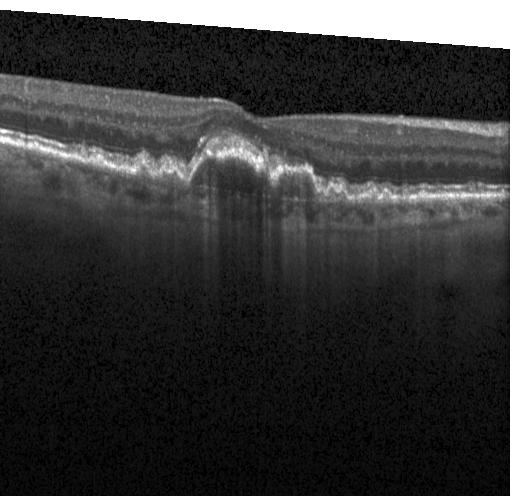
Optical coherence tomography scan; acquired on a Heidelberg Spectralis; macular scan — Finding: choroidal neovascularization (CNV).